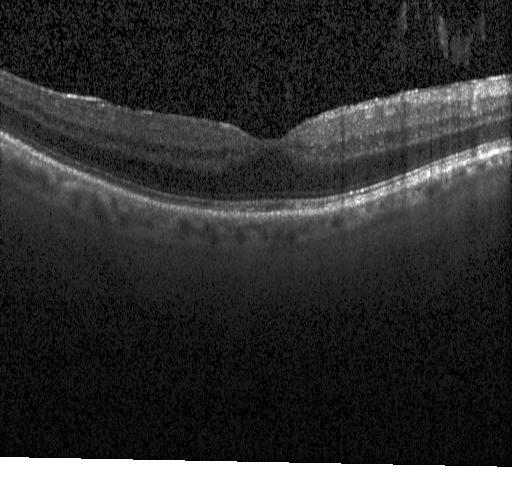 OCT B-scan. Horizontal scan through the fovea
Diagnosis: neither CNV, DME, nor drusen.